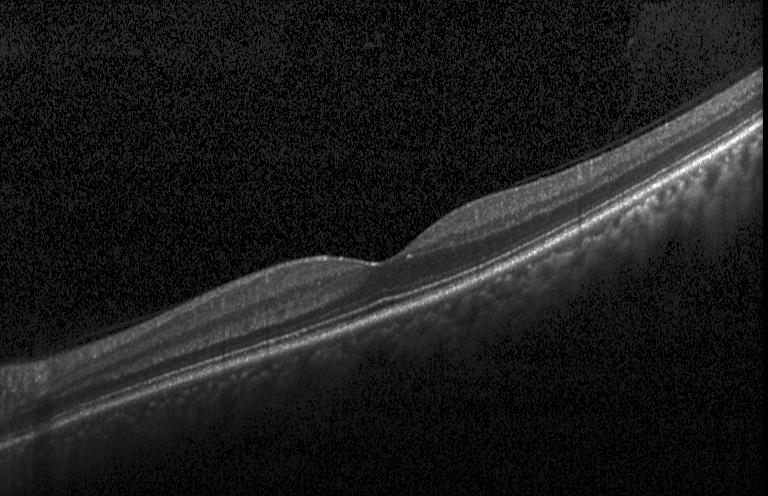

SD-OCT, optical coherence tomography B-scan, centered on the fovea.
Impression: no evidence of choroidal neovascularization, diabetic macular edema, or drusen.